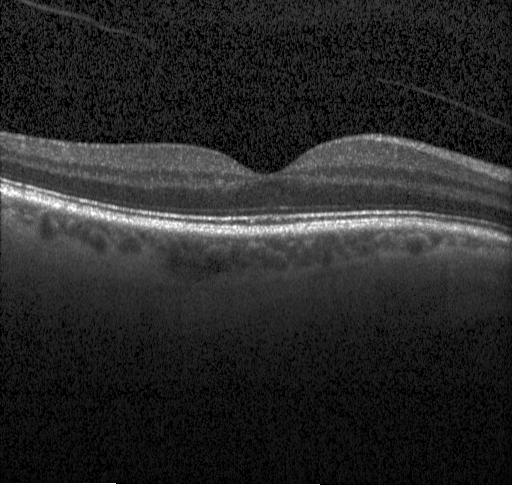
OCT B-scan showing no choroidal neovascularization, diabetic macular edema, or drusen.